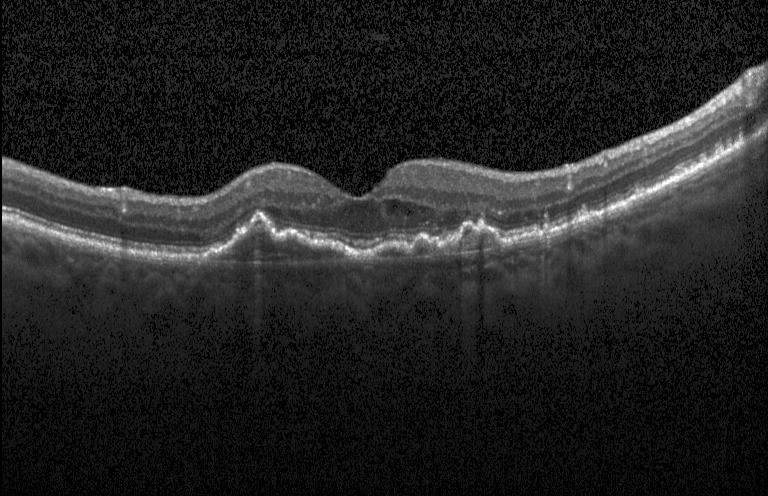
OCT B-scan — Diagnosis: a choroidal neovascular membrane.